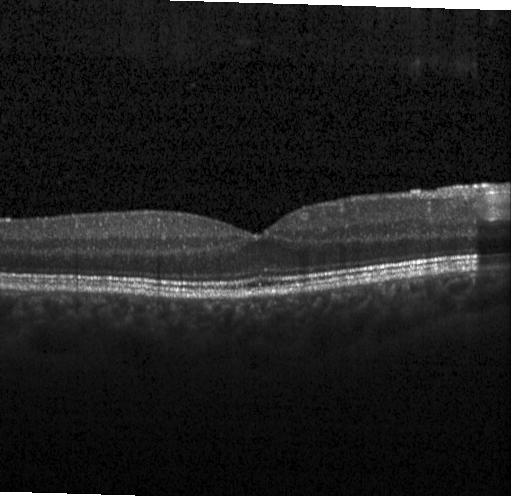

OCT B-scan showing no evidence of choroidal neovascularization, diabetic macular edema, or drusen.